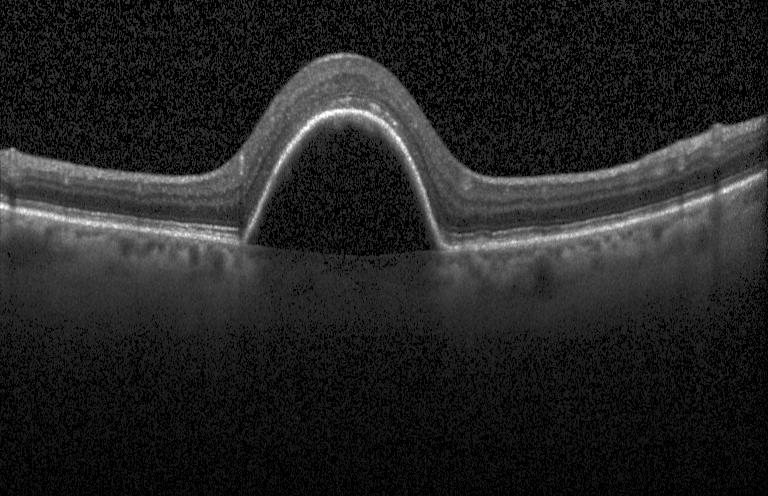
OCT line scan. Finding: CNV.